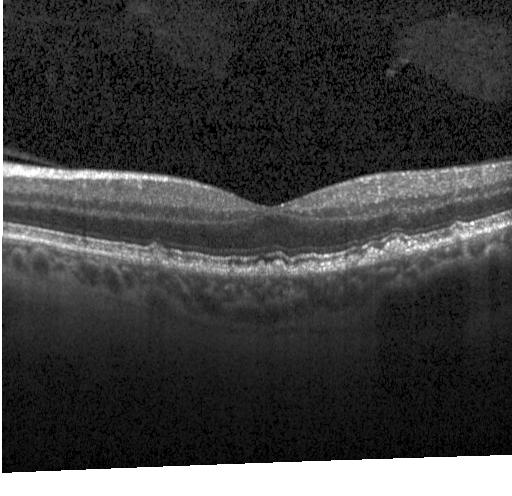
Heidelberg Spectralis · through the macula · retinal OCT cross-section.
Finding: multiple drusen.